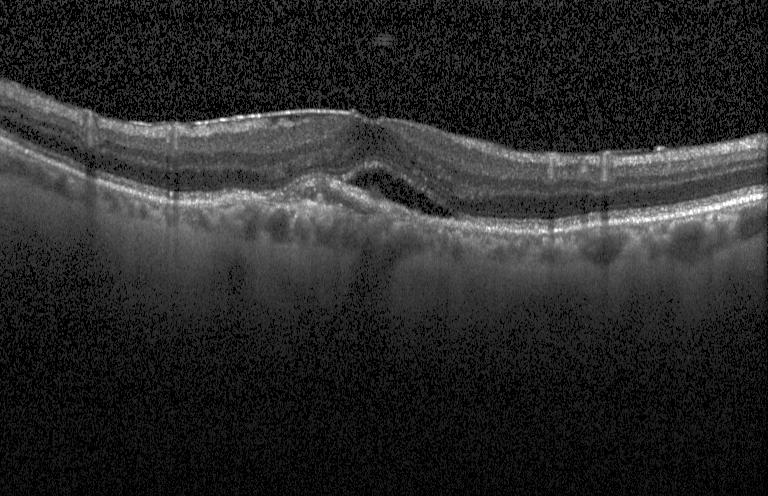 Diagnosis: a choroidal neovascular membrane.